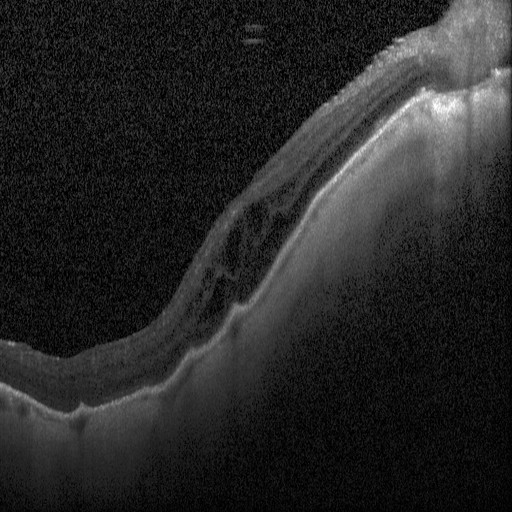 Fovea-centered; acquired on a Heidelberg Spectralis; SD-OCT; optical coherence tomography B-scan — Dx: diabetic macular edema.